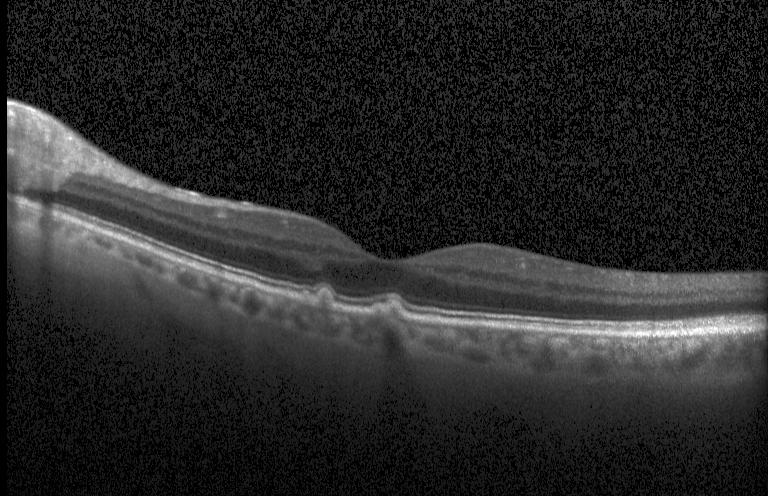

Through the macula; retinal OCT B-scan; Heidelberg Spectralis; spectral-domain optical coherence tomography.
This B-scan demonstrates drusen.